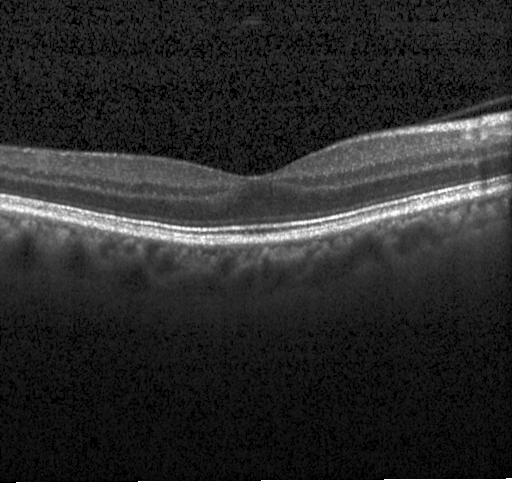
Macular scan · OCT B-scan · SD-OCT — Diagnosis: neither choroidal neovascularization, diabetic macular edema, nor drusen.